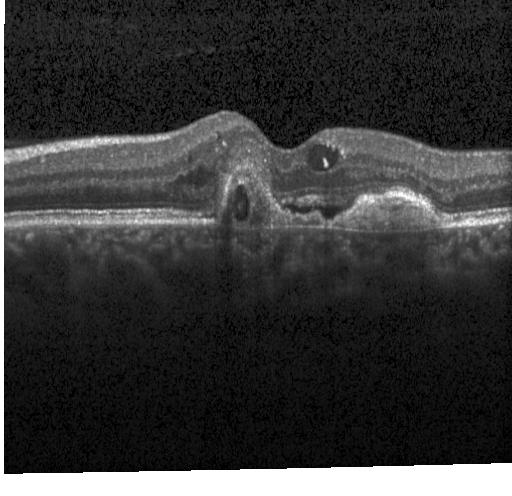 Diagnosis: choroidal neovascularization (CNV).